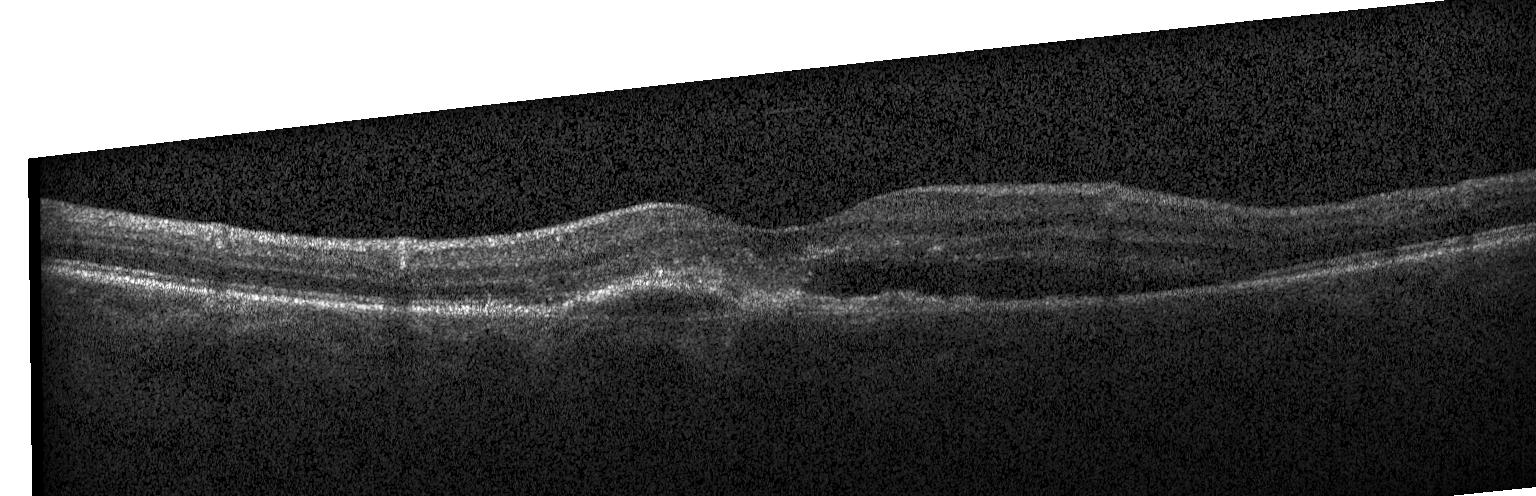
Diagnosis: a choroidal neovascular membrane.